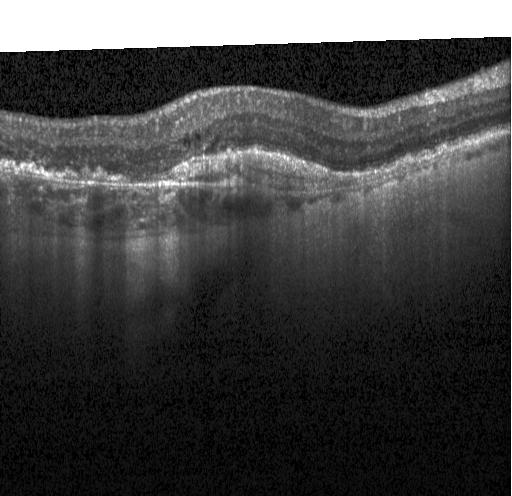

OCT finding: choroidal neovascularization.